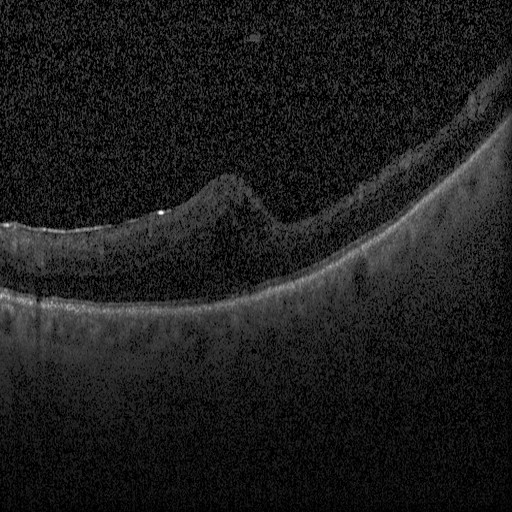 Retinal OCT cross-section showing diabetic macular edema (DME).